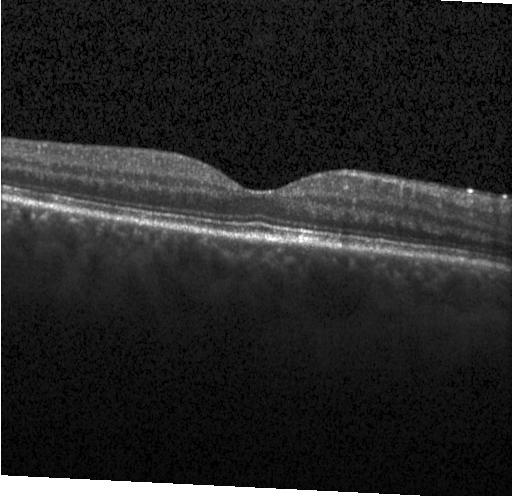
Optical coherence tomography scan · macular scan · SD-OCT.
The scan shows no choroidal neovascularization, no diabetic macular edema, and no drusen.